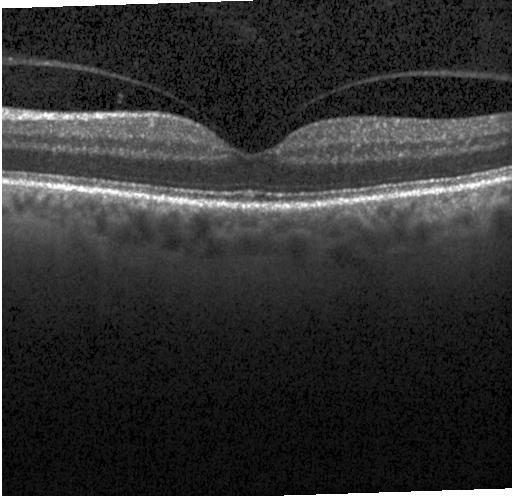
Acquired on a Heidelberg Spectralis; macular scan; optical coherence tomography B-scan
Impression: no choroidal neovascularization, no diabetic macular edema, and no drusen.